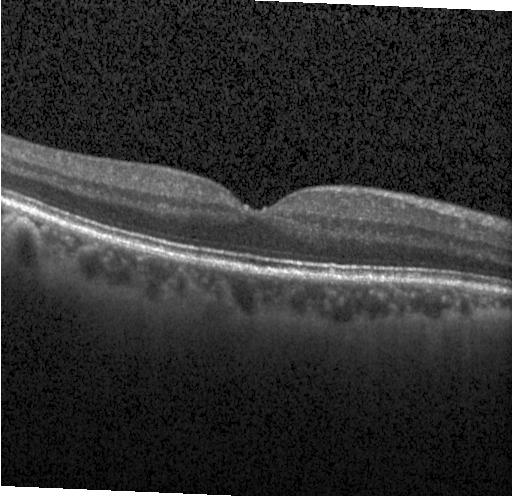
Heidelberg Spectralis OCT system. Retinal OCT cross-section. Diagnosis: neither choroidal neovascularization, diabetic macular edema, nor drusen.